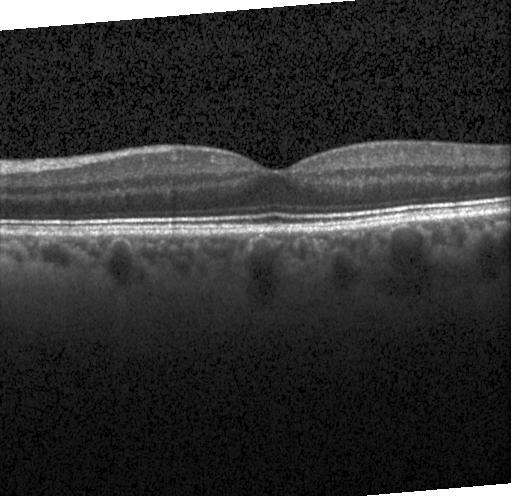

Acquired on a Heidelberg Spectralis · OCT B-scan.
Impression: neither CNV, DME, nor drusen.